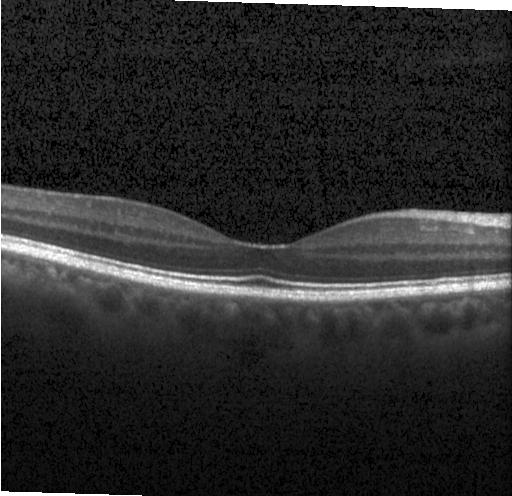 Dx: no evidence of CNV, DME, or drusen.